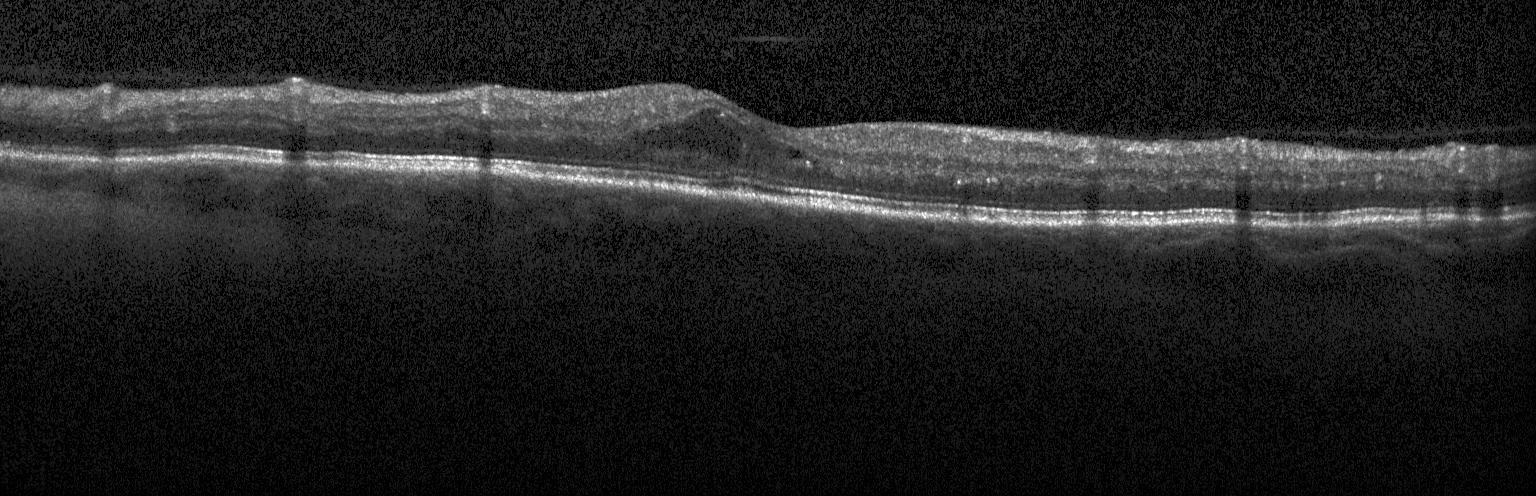
Dx: DME.